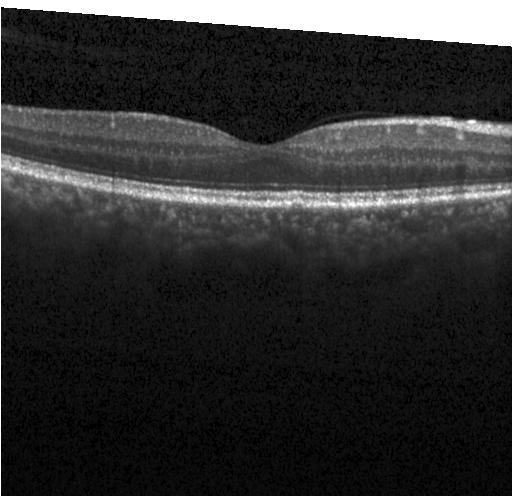
Retinal OCT B-scan; centered on the fovea — The scan shows no evidence of choroidal neovascularization, diabetic macular edema, or drusen.